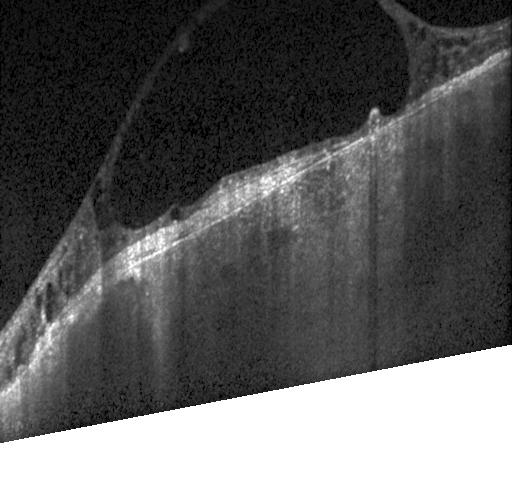 Heidelberg Spectralis OCT system; OCT B-scan; fovea-centered. The scan shows a choroidal neovascular membrane.